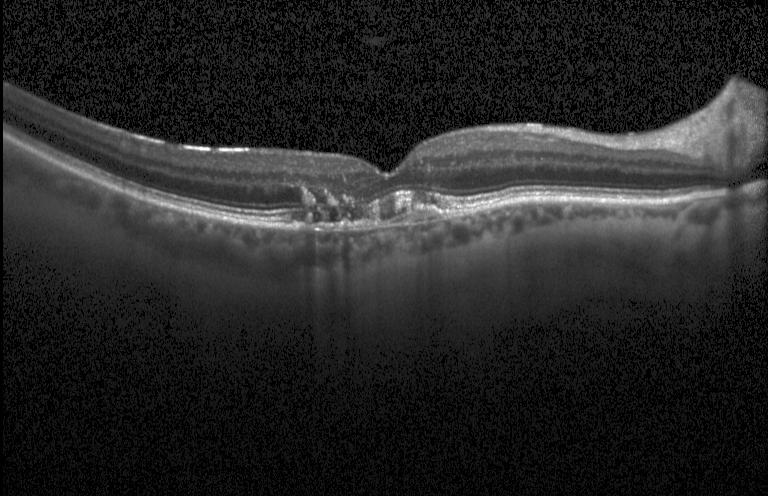 Spectral-domain OCT, OCT B-scan, through the macula, Heidelberg Spectralis OCT system — Impression: choroidal neovascularization.